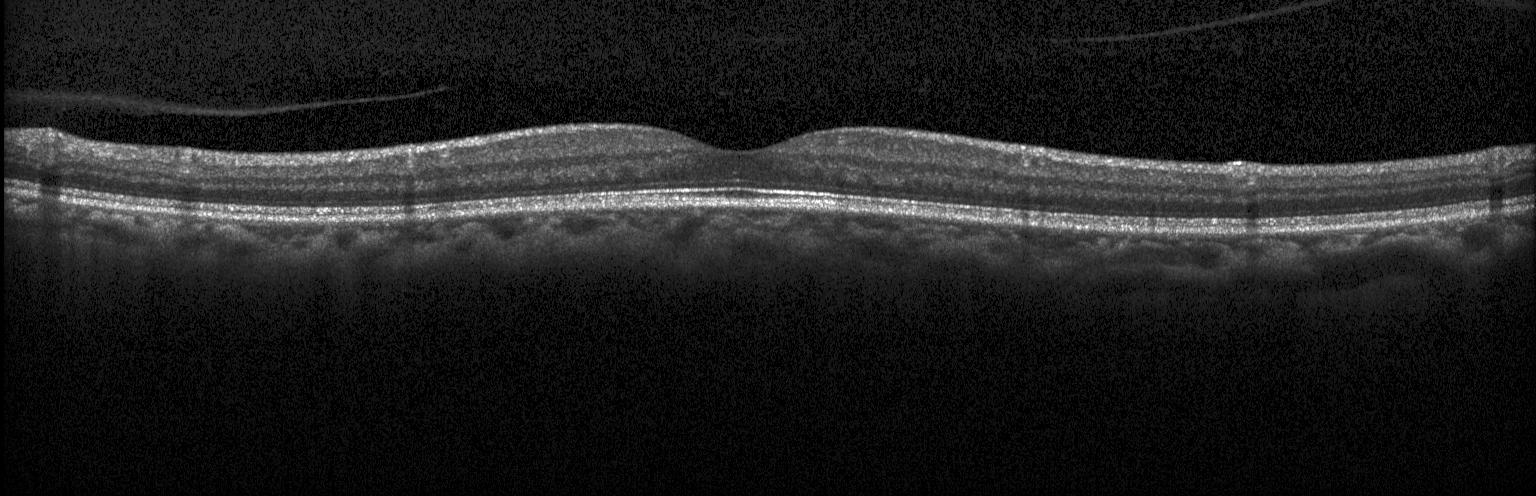

Macular scan, retinal OCT B-scan, acquired on a Heidelberg Spectralis. Macular OCT: no choroidal neovascularization, no diabetic macular edema, and no drusen.